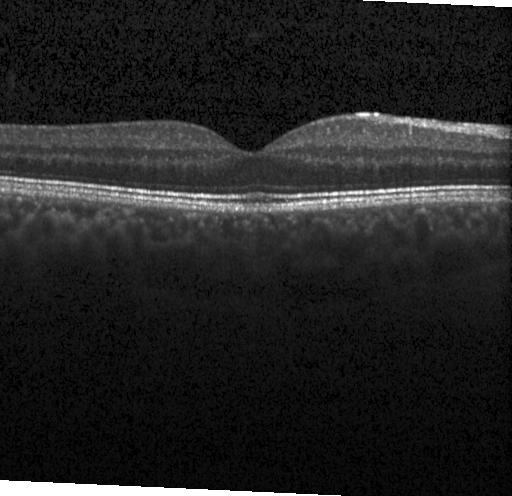

Optical coherence tomography B-scan — Diagnosis: neither CNV, DME, nor drusen.